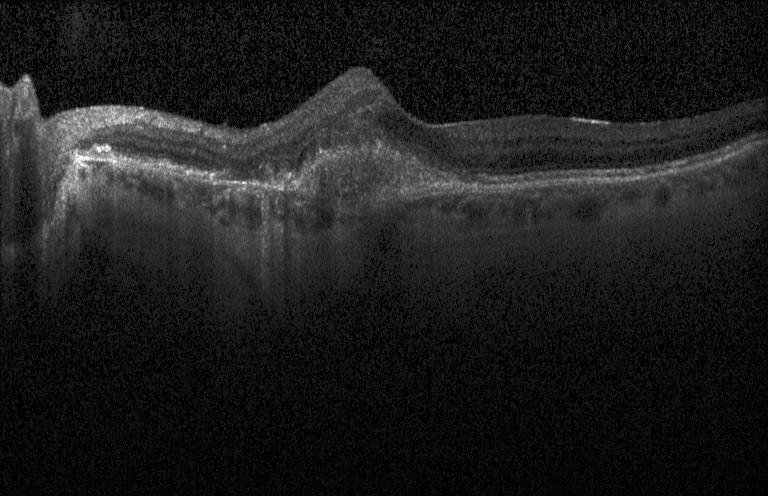
OCT finding: CNV.